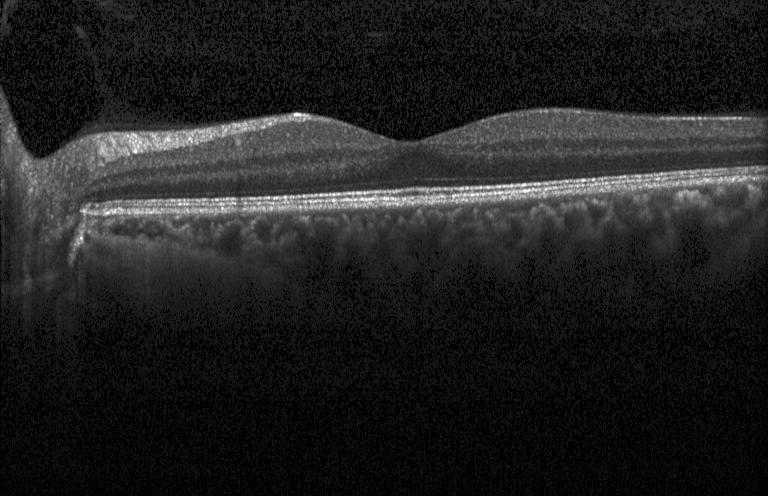

Horizontal scan through the fovea. OCT line scan. Heidelberg Spectralis
Diagnosis: no choroidal neovascularization, no diabetic macular edema, and no drusen.